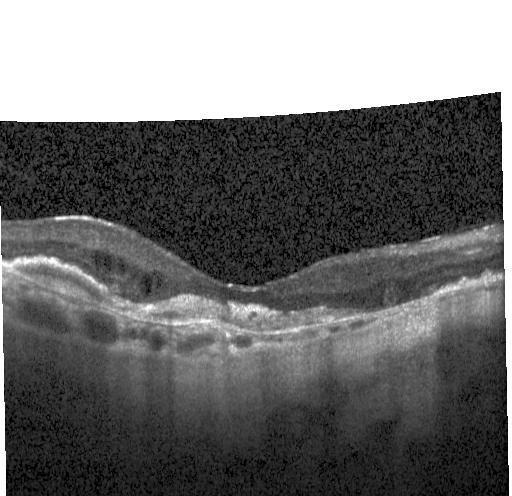

Heidelberg Spectralis · SD-OCT · optical coherence tomography scan. Diagnosis: CNV.